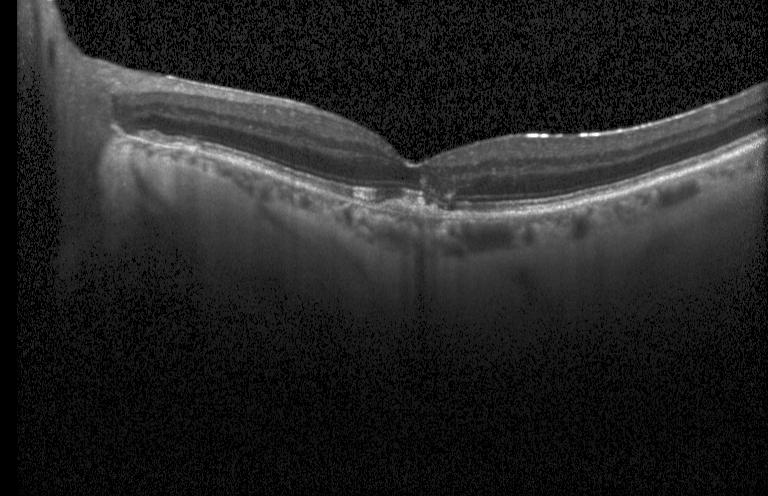
Fovea-centered; optical coherence tomography B-scan; spectral-domain optical coherence tomography; instrument: Heidelberg Spectralis.
Dx: a choroidal neovascular membrane.